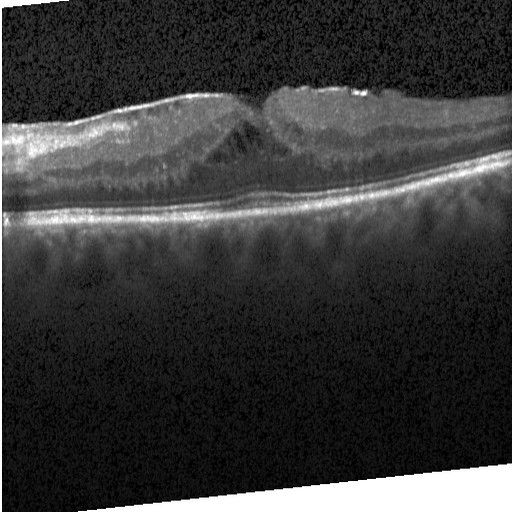
Spectral-domain optical coherence tomography, OCT B-scan
The scan shows DME.